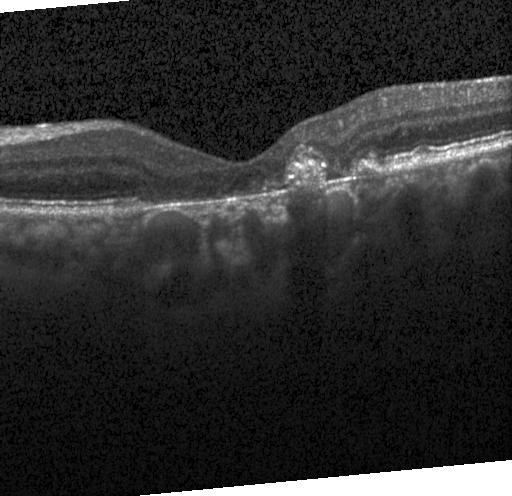
Retinal OCT B-scan. OCT finding: a choroidal neovascular membrane.